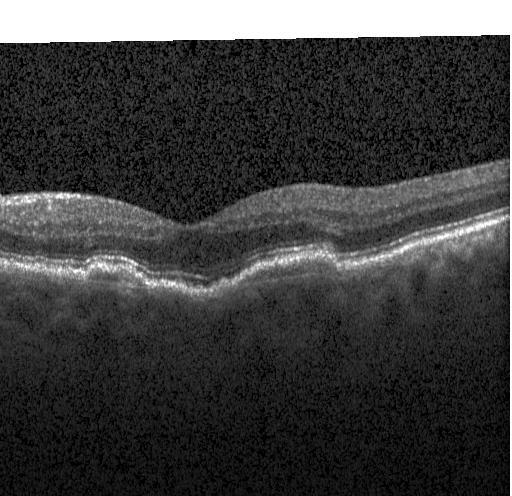

OCT B-scan. SD-OCT. Centered on the fovea.
Impression: a choroidal neovascular membrane.